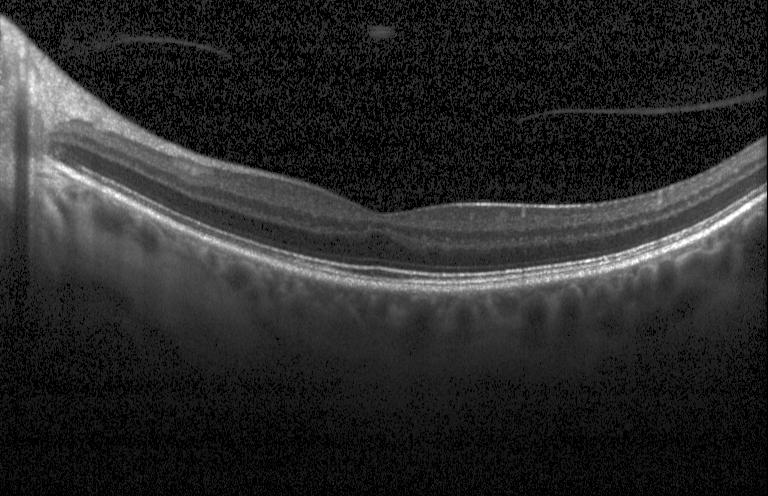 Retinal OCT cross-section.
Dx: no evidence of choroidal neovascularization, diabetic macular edema, or drusen.